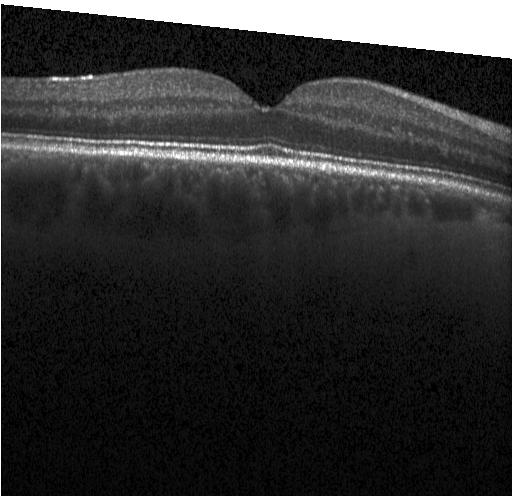

Diagnosis: no choroidal neovascularization, diabetic macular edema, or drusen.